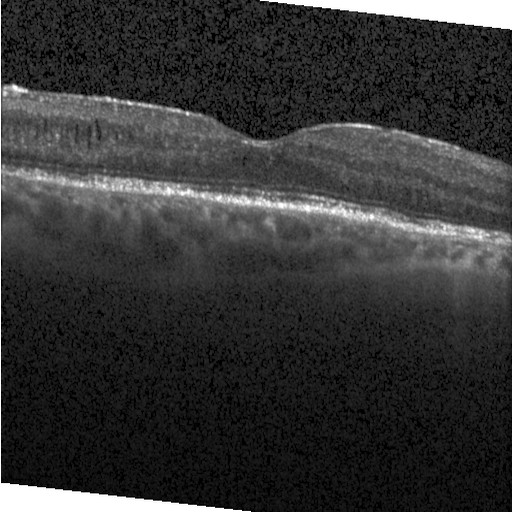 Centered on the fovea. SD-OCT. Optical coherence tomography scan. Acquired on a Heidelberg Spectralis. Dx: diabetic macular edema (DME).